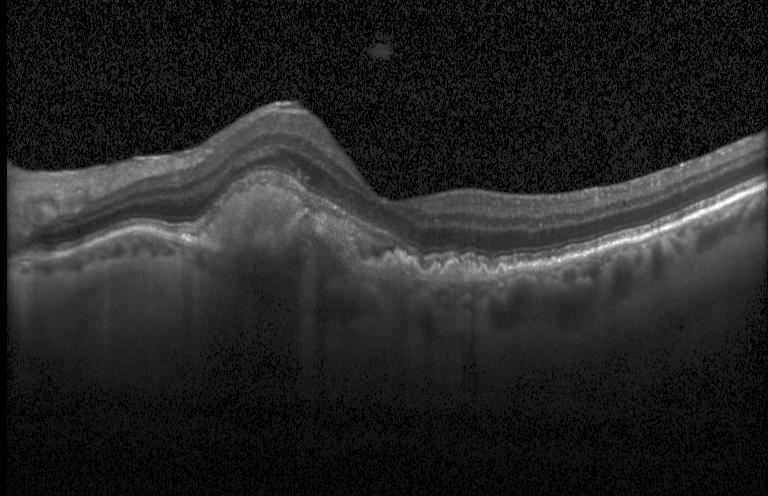

Horizontal scan through the fovea, Heidelberg Spectralis, retinal OCT cross-section.
Impression: choroidal neovascularization.